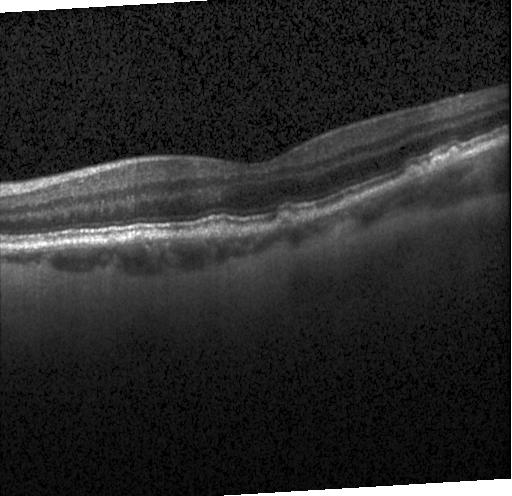

OCT B-scan; through the macula. Finding: drusen.